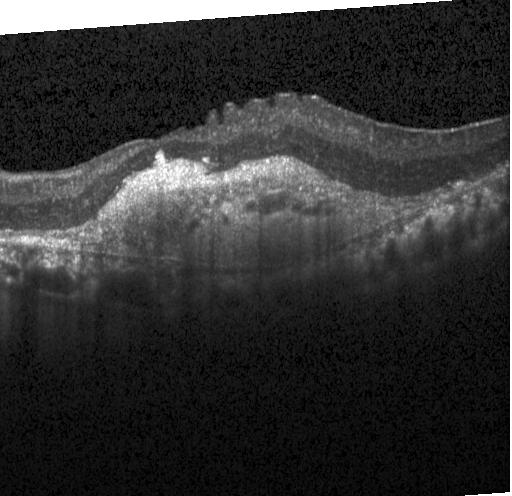 Horizontal scan through the fovea · Heidelberg Spectralis · retinal OCT cross-section · spectral-domain optical coherence tomography — Macular OCT: a choroidal neovascular membrane.